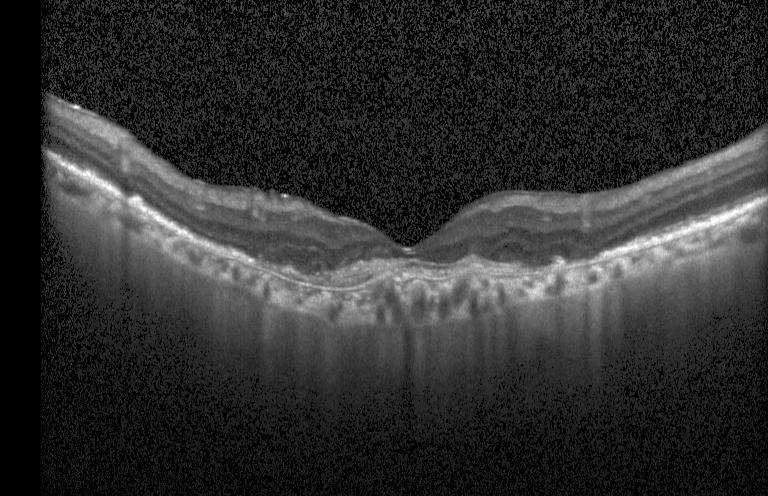

Retinal OCT cross-section showing choroidal neovascularization (CNV).